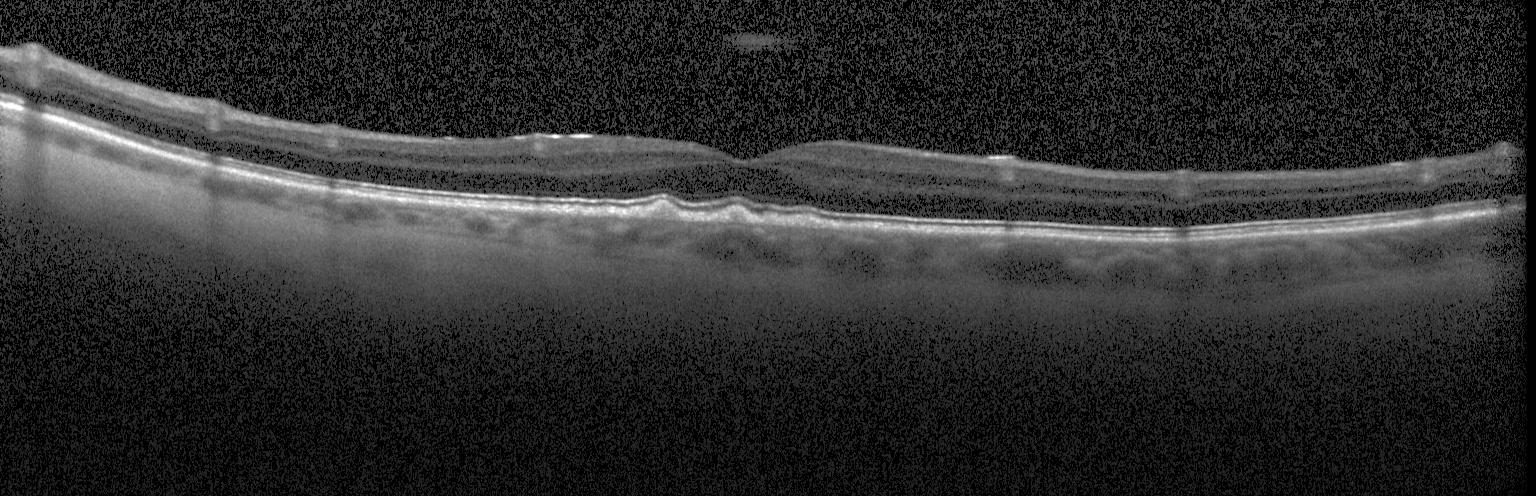
Optical coherence tomography scan. Finding: drusen.